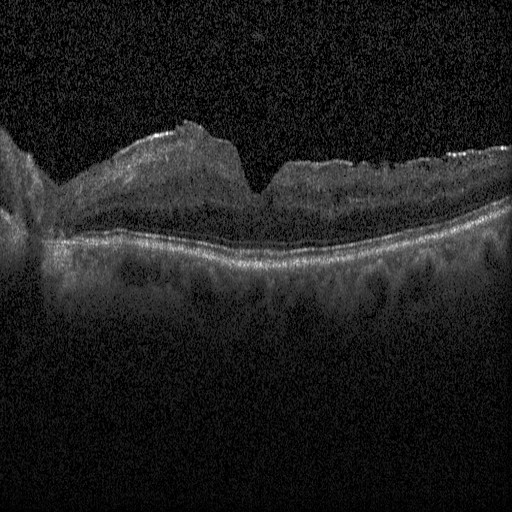

Instrument: Heidelberg Spectralis · spectral-domain OCT · horizontal scan through the fovea · retinal OCT cross-section — DME.